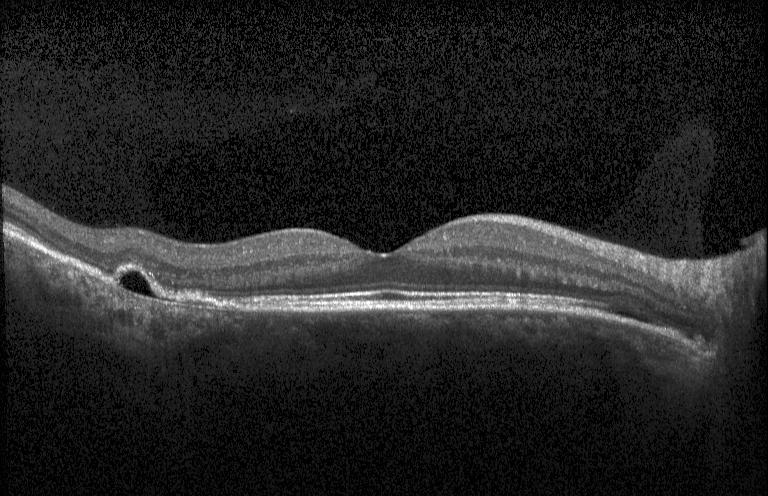

Optical coherence tomography B-scan. Finding: choroidal neovascularization.